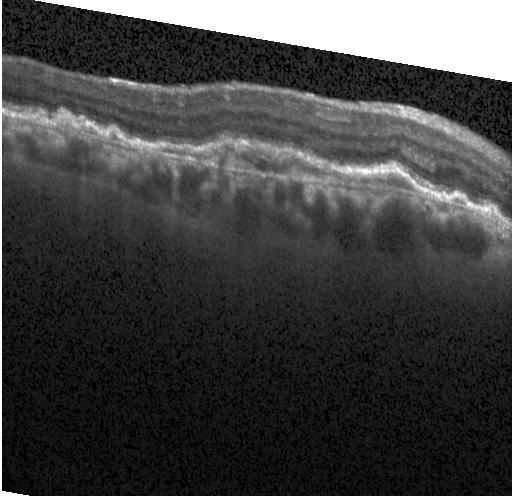 Fovea-centered · OCT B-scan · Heidelberg Spectralis OCT system · spectral-domain optical coherence tomography
Finding: choroidal neovascularization (CNV).